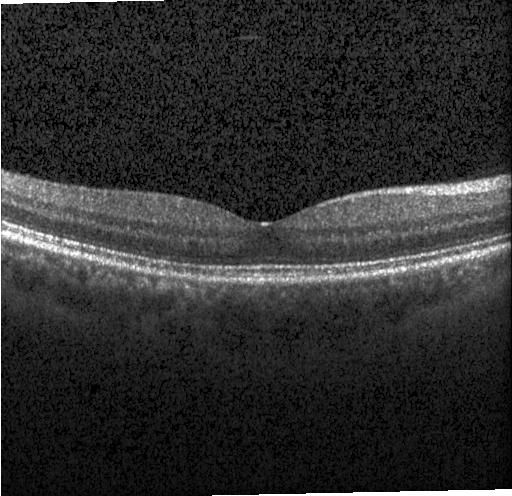 Instrument: Heidelberg Spectralis · retinal OCT B-scan · spectral-domain optical coherence tomography. Diagnosis: neither choroidal neovascularization, diabetic macular edema, nor drusen.